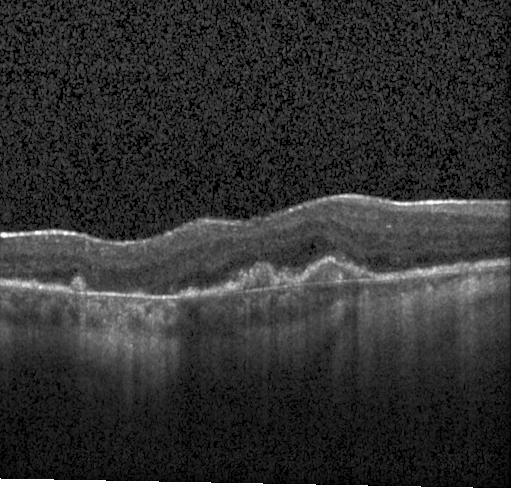
Retinal OCT B-scan.
This B-scan demonstrates a choroidal neovascular membrane.